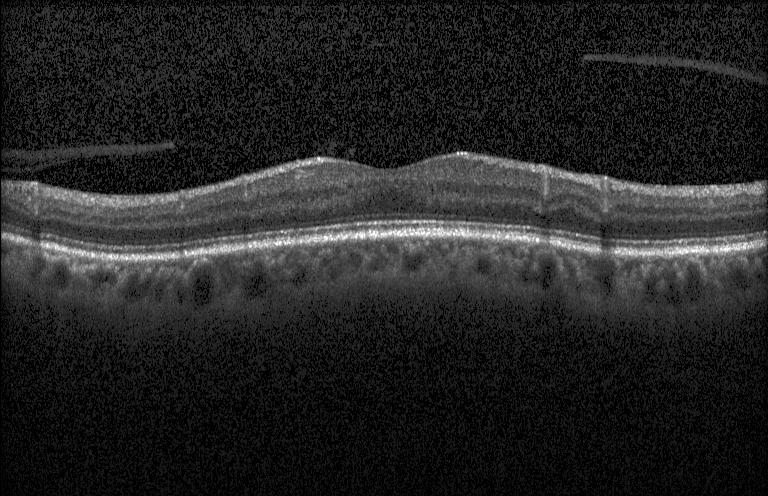

Macular scan, spectral-domain OCT, retinal OCT cross-section, Heidelberg Spectralis
The scan shows no evidence of choroidal neovascularization, diabetic macular edema, or drusen.